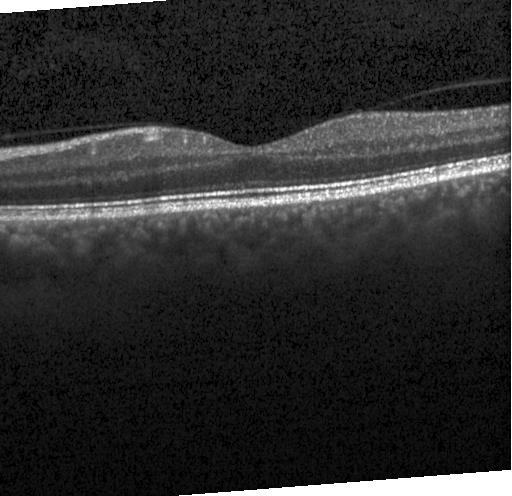 Optical coherence tomography scan · Heidelberg Spectralis OCT system · spectral-domain optical coherence tomography
Finding: no choroidal neovascularization, diabetic macular edema, or drusen.